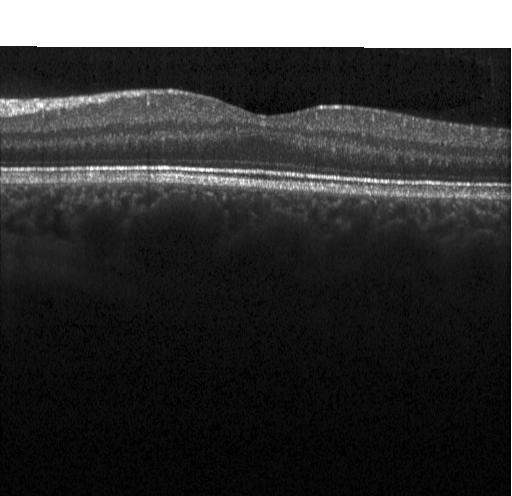
Through the macula; Heidelberg Spectralis OCT system; optical coherence tomography B-scan
Impression: neither CNV, DME, nor drusen.